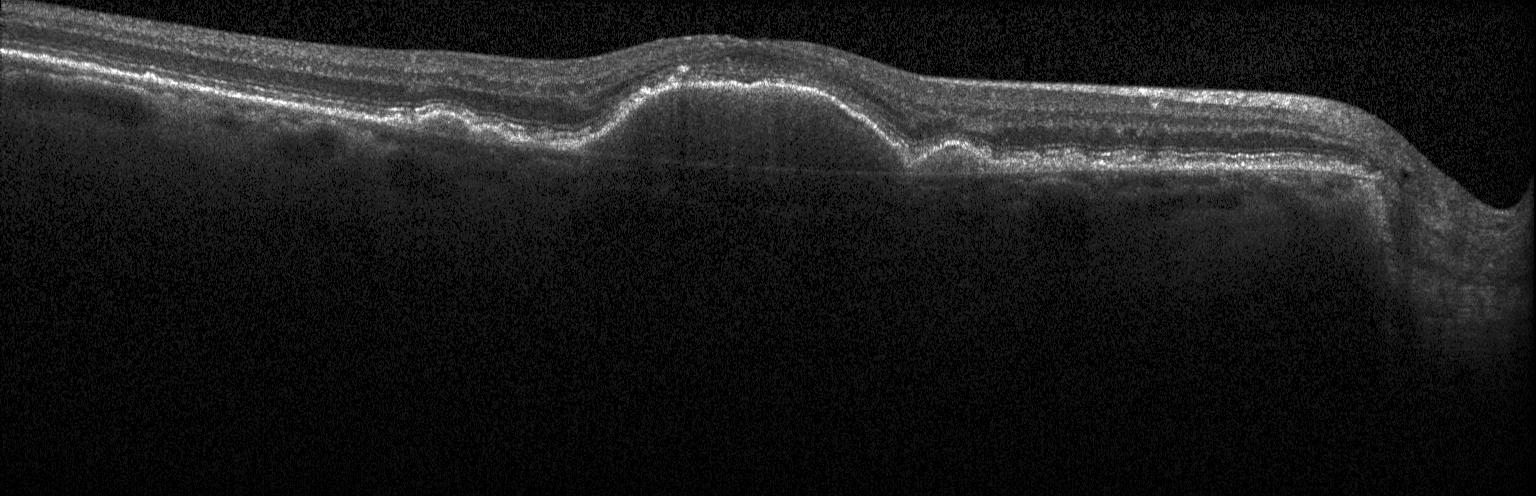

Optical coherence tomography scan; through the macula; instrument: Heidelberg Spectralis; spectral-domain OCT — Diagnosis: a choroidal neovascular membrane.